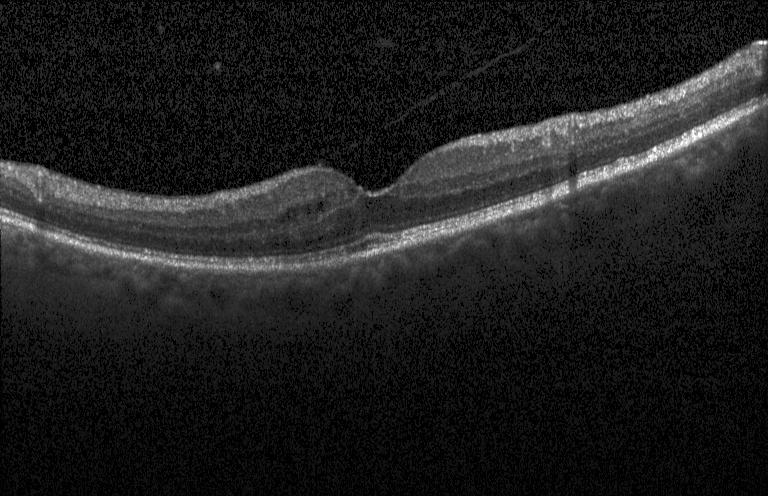

Spectral-domain OCT B-scan: diabetic macular edema (DME).